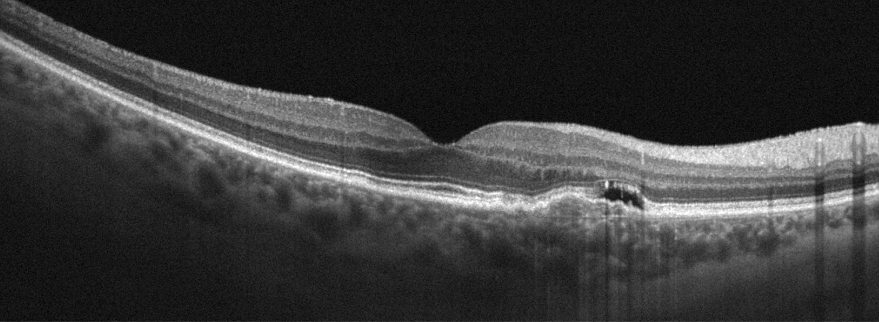

Retinal OCT B-scan. Finding: age-related macular degeneration (AMD).